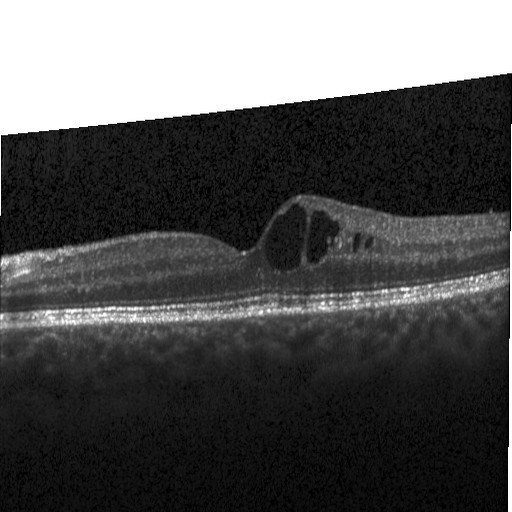

Centered on the fovea. Spectral-domain OCT. Optical coherence tomography scan. Heidelberg Spectralis OCT system — Finding: diabetic macular edema.